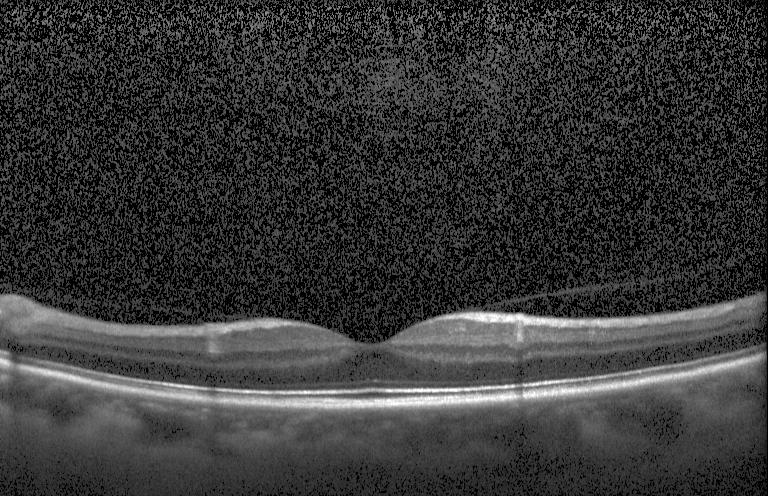 Optical coherence tomography B-scan; horizontal scan through the fovea
Dx: no CNV, DME, or drusen.